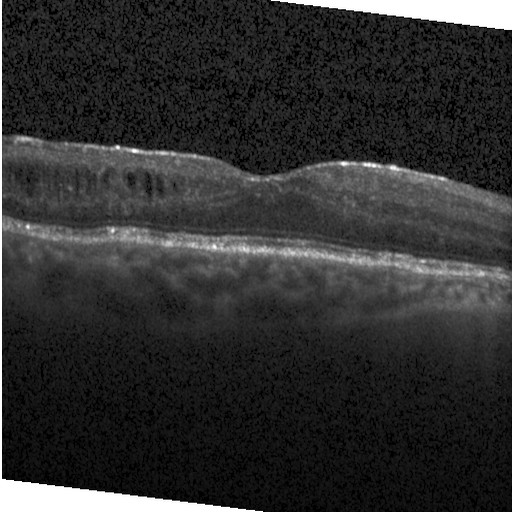
OCT finding: DME.